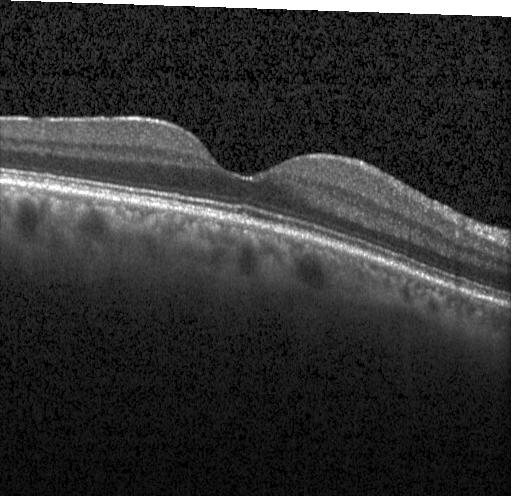 The scan shows no choroidal neovascularization, diabetic macular edema, or drusen.